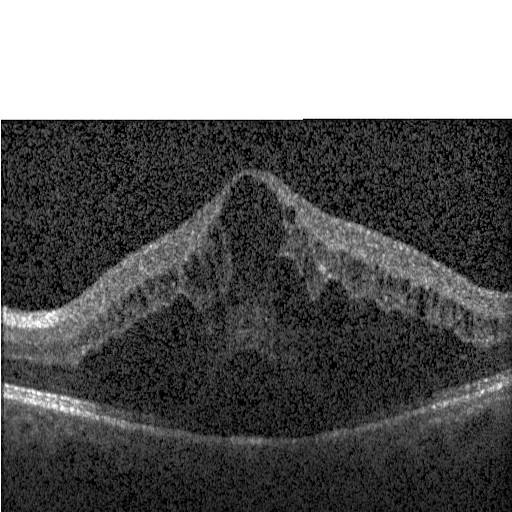
Retinal OCT cross-section, Heidelberg Spectralis OCT system.
The scan shows DME.